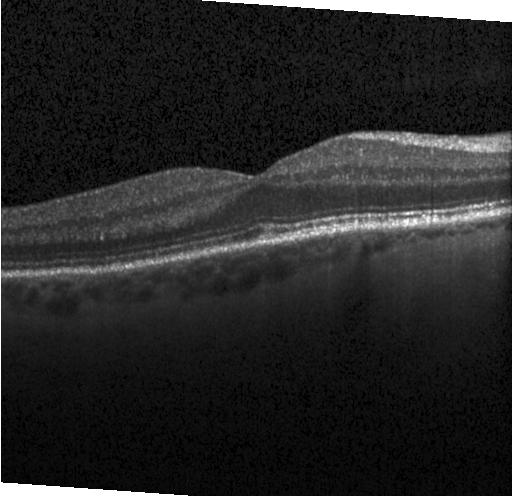
Fovea-centered · optical coherence tomography B-scan · acquired on a Heidelberg Spectralis — OCT finding: neither choroidal neovascularization, diabetic macular edema, nor drusen.